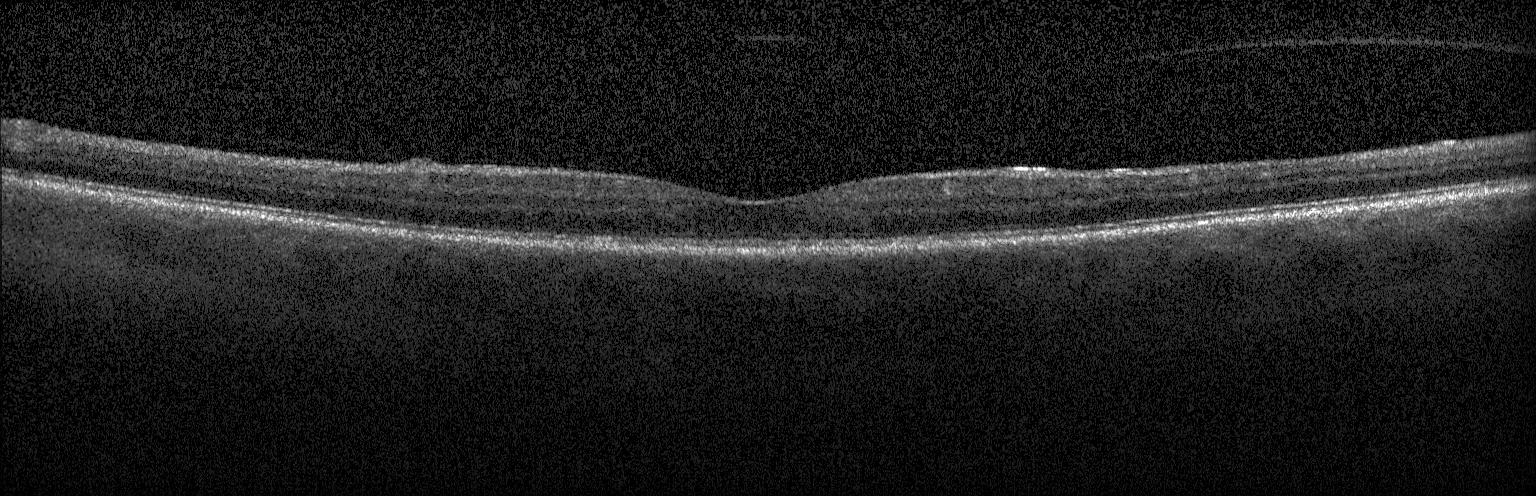 Neither choroidal neovascularization, diabetic macular edema, nor drusen.